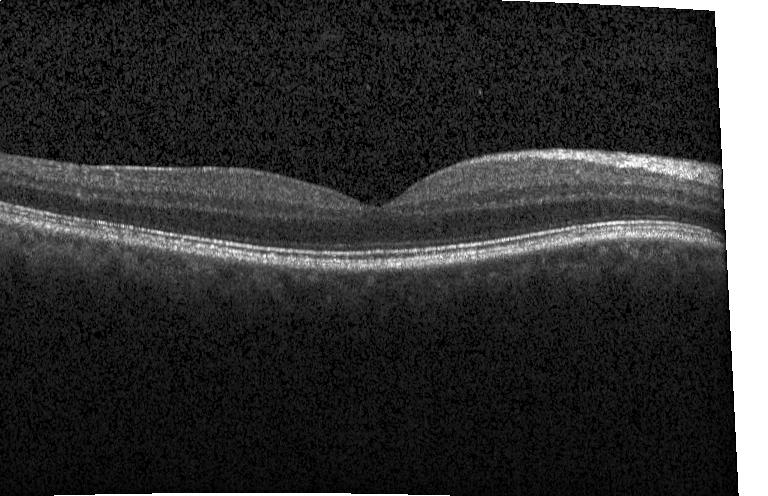
Spectral-domain OCT B-scan: no choroidal neovascularization, diabetic macular edema, or drusen.